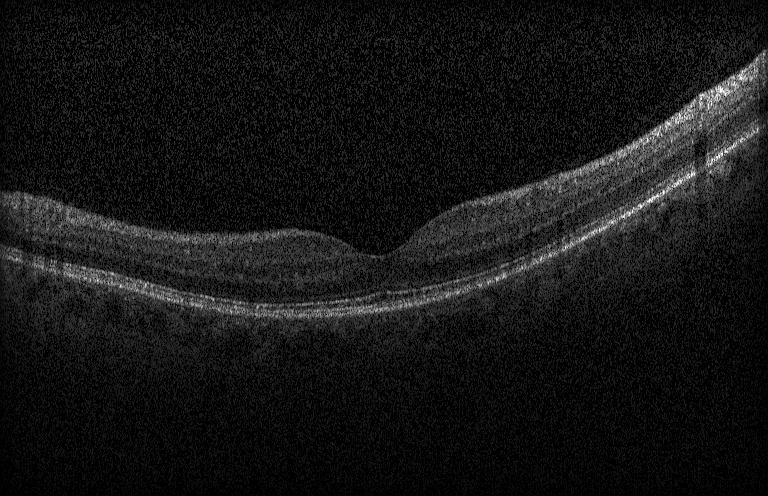

Instrument: Heidelberg Spectralis · optical coherence tomography B-scan.
OCT finding: neither CNV, DME, nor drusen.